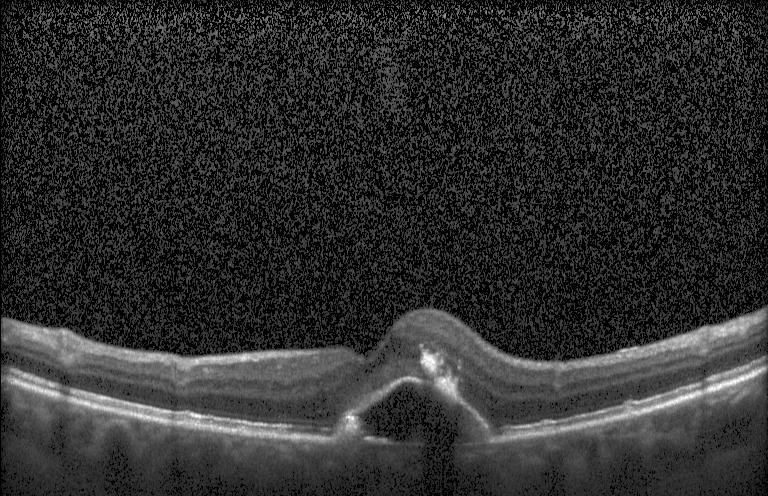
Instrument: Heidelberg Spectralis; SD-OCT; optical coherence tomography B-scan; through the macula.
Macular OCT: a choroidal neovascular membrane.